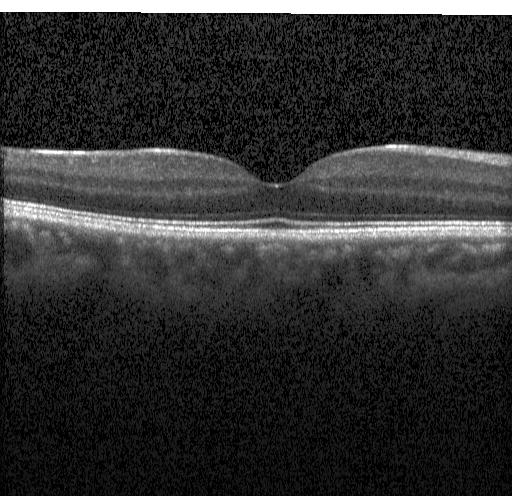
Optical coherence tomography B-scan.
The scan shows neither choroidal neovascularization, diabetic macular edema, nor drusen.